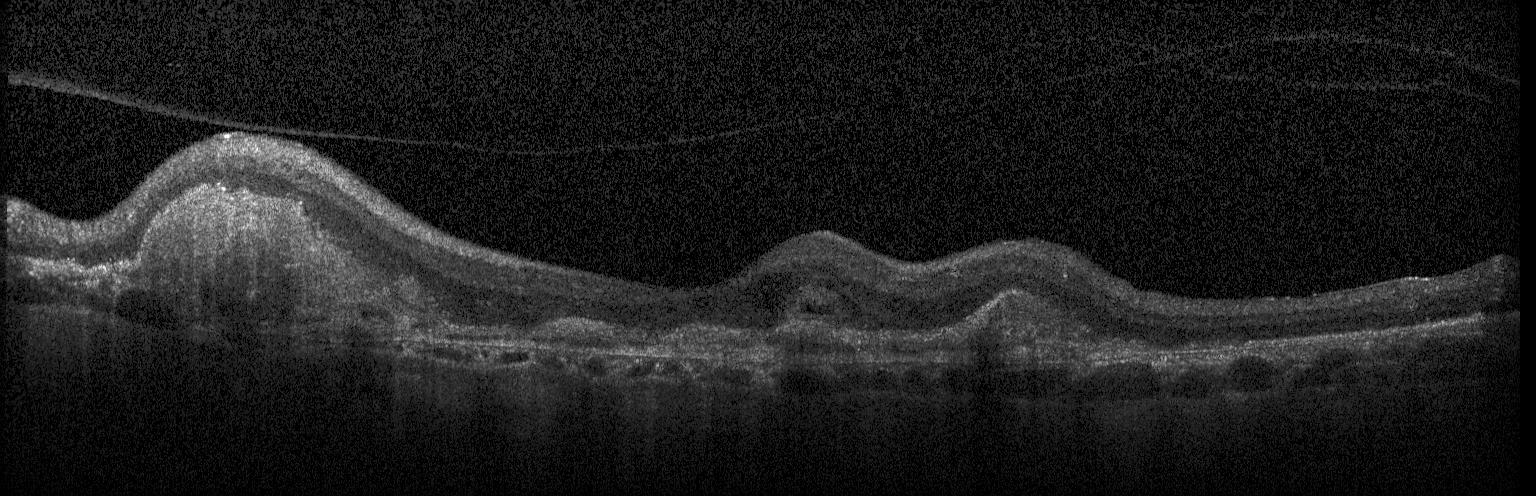 Optical coherence tomography B-scan. Spectral-domain OCT. Acquired on a Heidelberg Spectralis
This B-scan demonstrates a choroidal neovascular membrane.